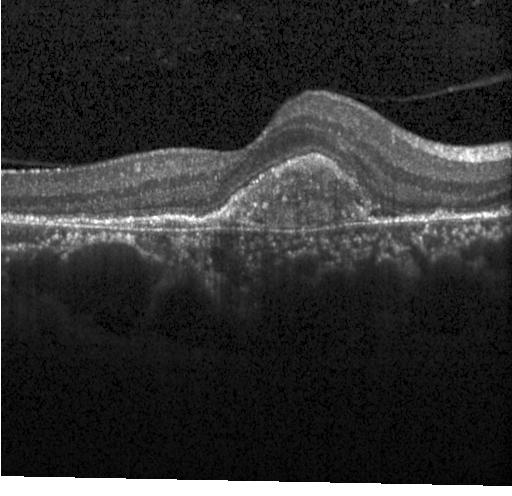

Dx: a choroidal neovascular membrane.